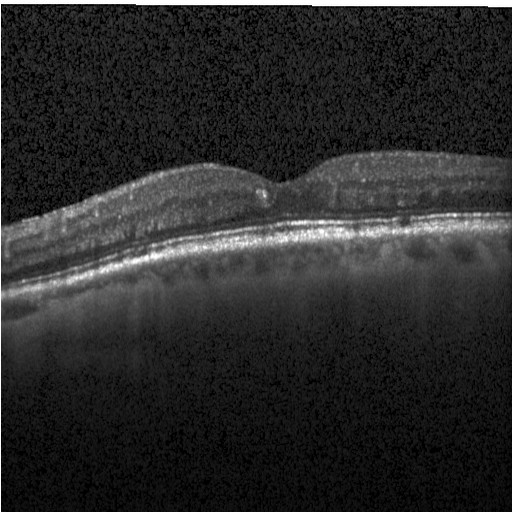

Acquired on a Heidelberg Spectralis, retinal OCT cross-section, macular scan, spectral-domain OCT.
Diagnosis: diabetic macular edema (DME).